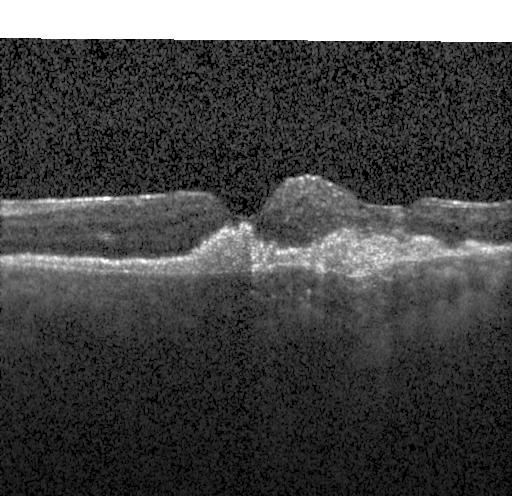
OCT line scan.
Macular OCT: choroidal neovascularization (CNV).